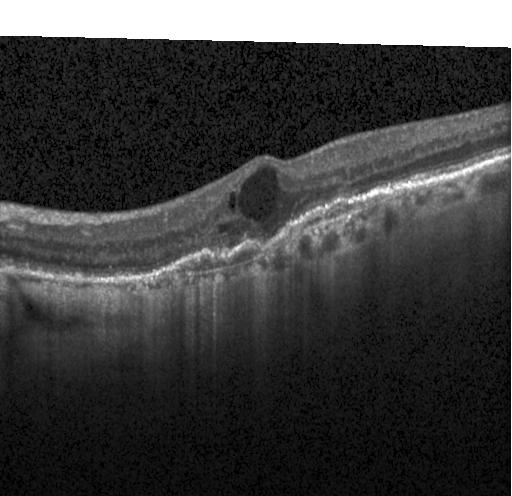
OCT B-scan; through the macula; SD-OCT
Diagnosis: choroidal neovascularization (CNV).